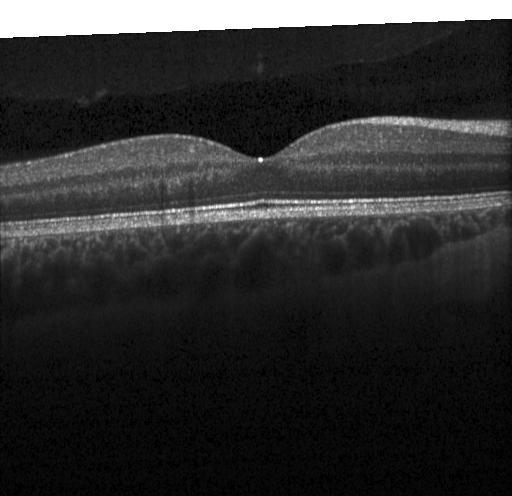
Fovea-centered, spectral-domain optical coherence tomography, OCT line scan
Diagnosis: no evidence of choroidal neovascularization, diabetic macular edema, or drusen.